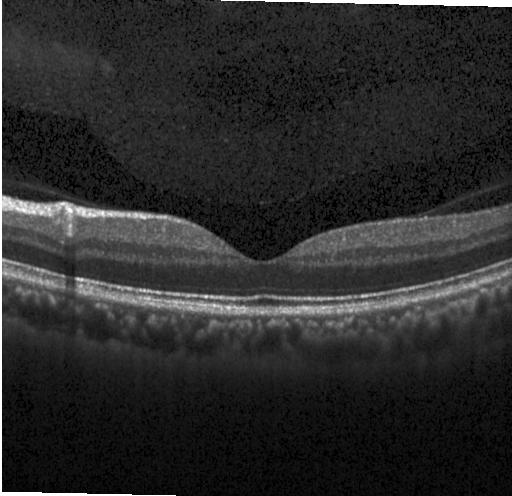

Macular OCT: no choroidal neovascularization, no diabetic macular edema, and no drusen.